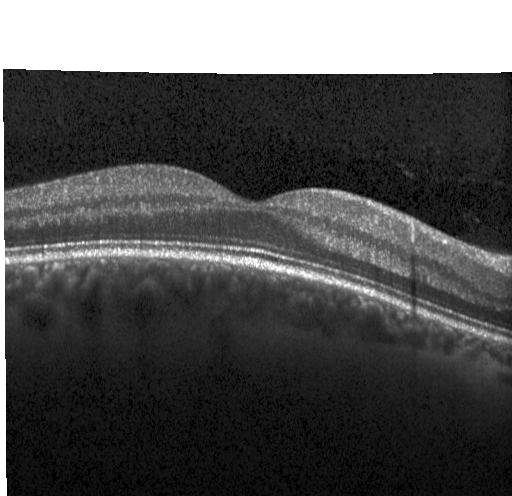 OCT B-scan, fovea-centered, spectral-domain optical coherence tomography — The scan shows no choroidal neovascularization, no diabetic macular edema, and no drusen.